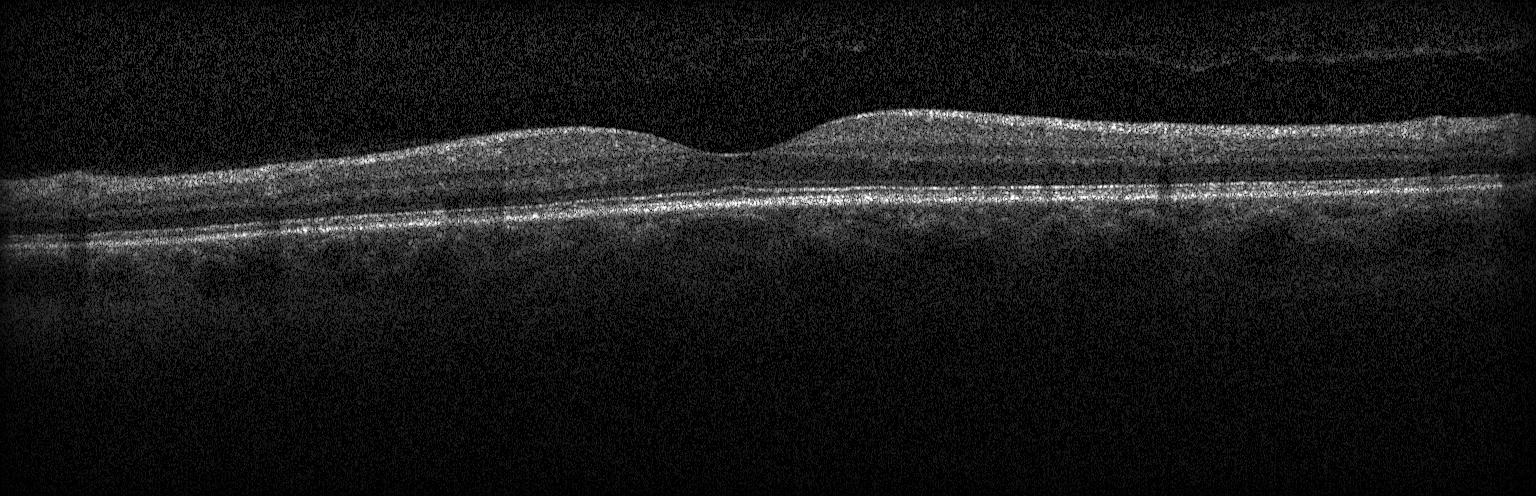
Retinal OCT B-scan — Dx: no evidence of choroidal neovascularization, diabetic macular edema, or drusen.